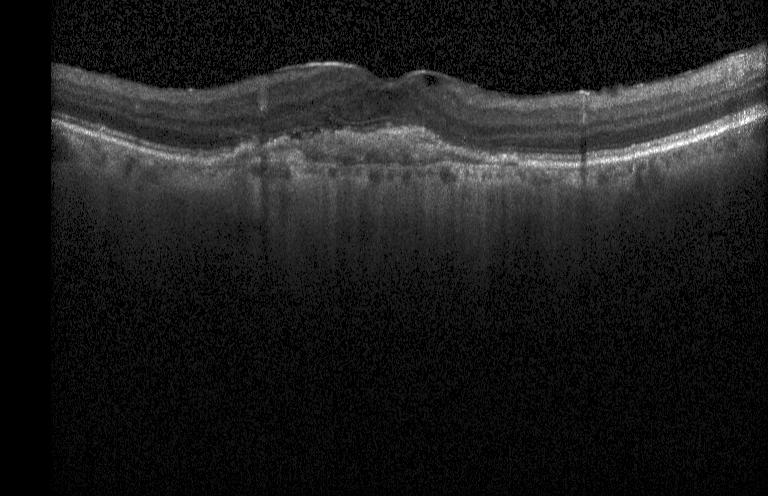
Spectral-domain OCT B-scan: a choroidal neovascular membrane.